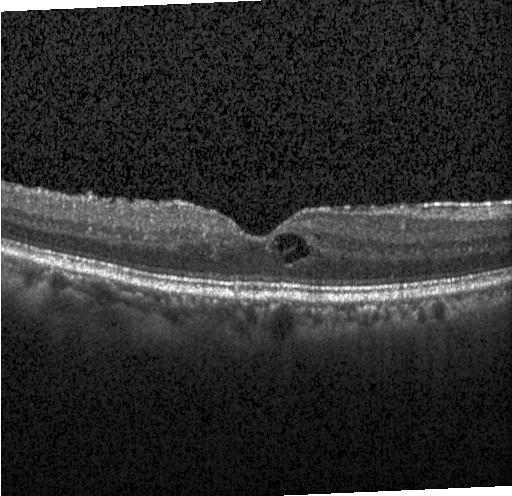
Impression: diabetic macular edema (DME).